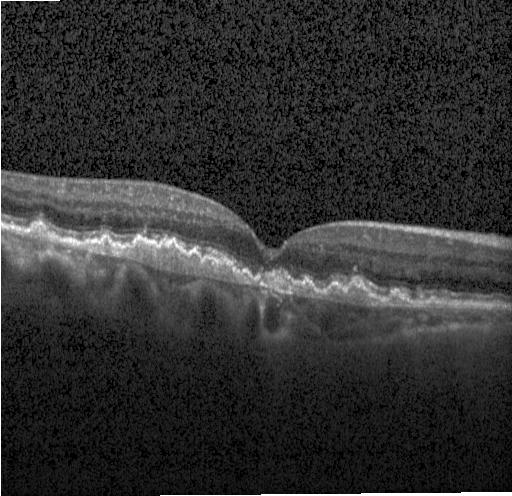

Impression: choroidal neovascularization (CNV).